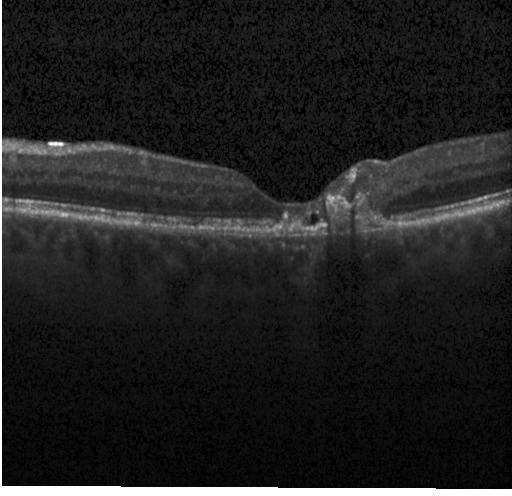 Retinal OCT cross-section.
Diagnosis: a choroidal neovascular membrane.